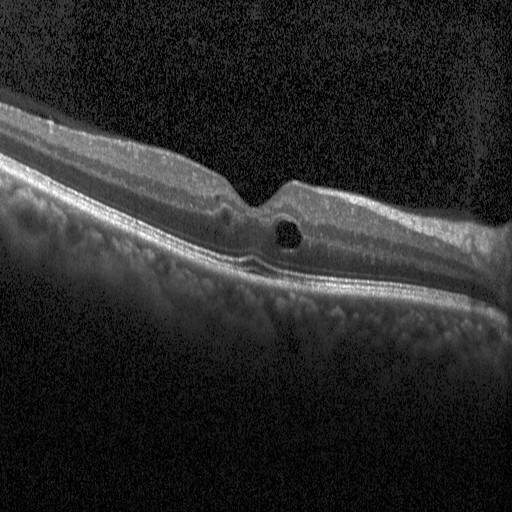
Fovea-centered · OCT line scan · acquired on a Heidelberg Spectralis · spectral-domain optical coherence tomography.
Diagnosis: DME.